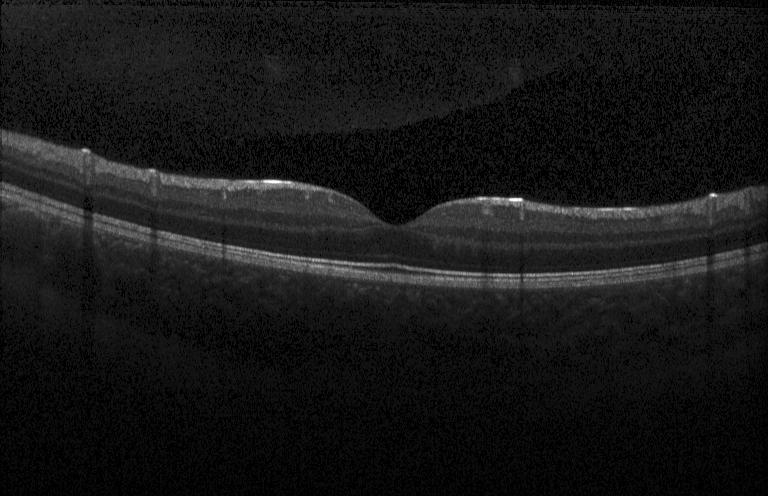
Impression: no evidence of CNV, DME, or drusen.